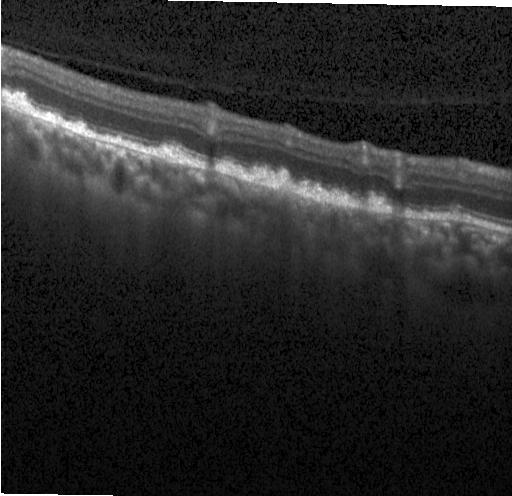 Finding: sub-RPE drusenoid deposits.